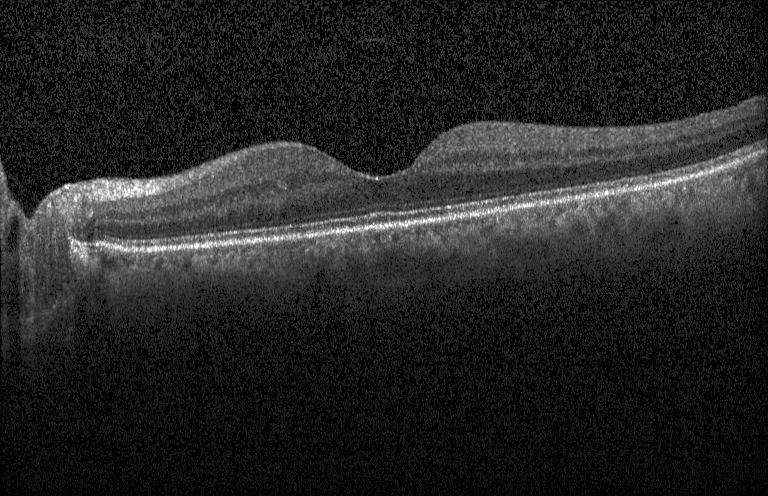

Retinal OCT cross-section · fovea-centered — No evidence of choroidal neovascularization, diabetic macular edema, or drusen.